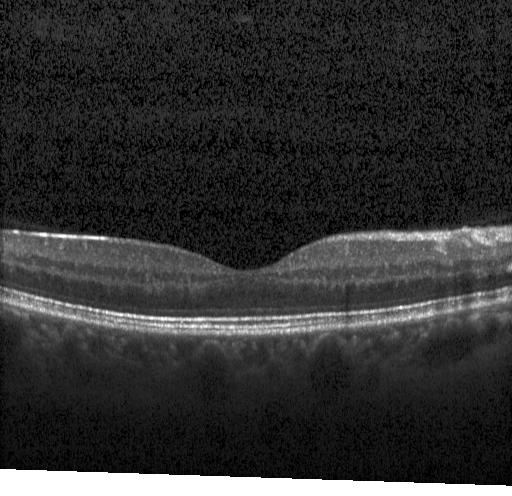
Horizontal scan through the fovea · retinal OCT B-scan · instrument: Heidelberg Spectralis · spectral-domain OCT
Assessment: no evidence of choroidal neovascularization, diabetic macular edema, or drusen.